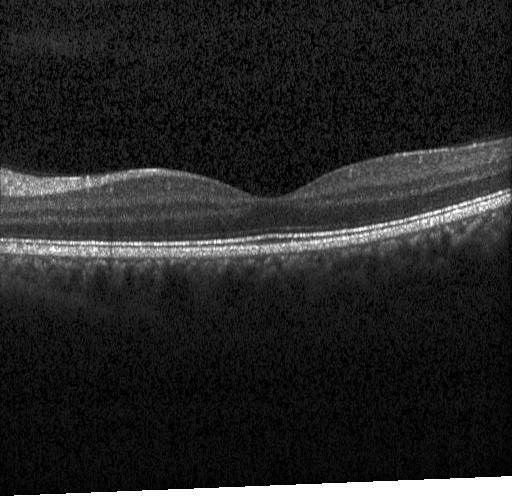

Heidelberg Spectralis · fovea-centered · OCT line scan — Finding: no evidence of CNV, DME, or drusen.